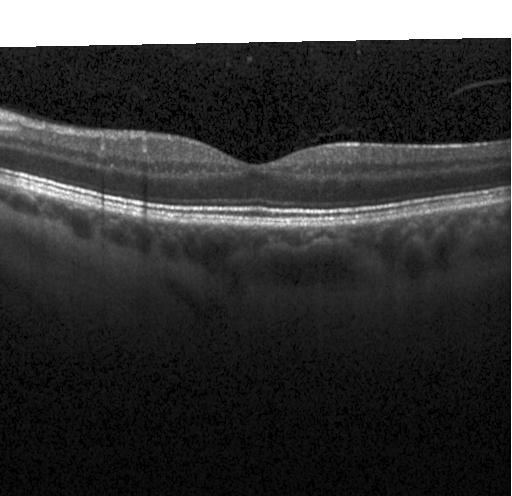
OCT line scan; spectral-domain OCT
The scan shows no CNV, DME, or drusen.